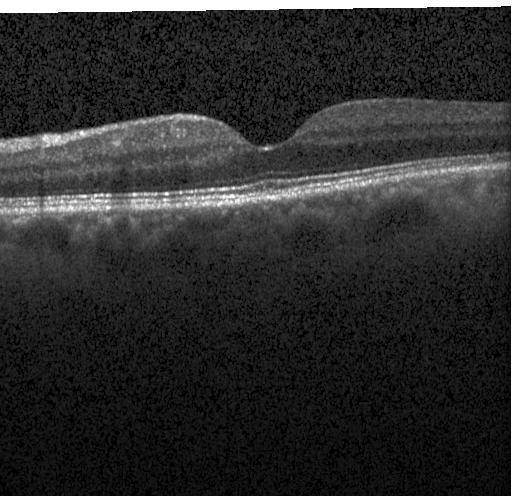
Through the macula · SD-OCT · acquired on a Heidelberg Spectralis · OCT B-scan
Finding: no choroidal neovascularization, diabetic macular edema, or drusen.